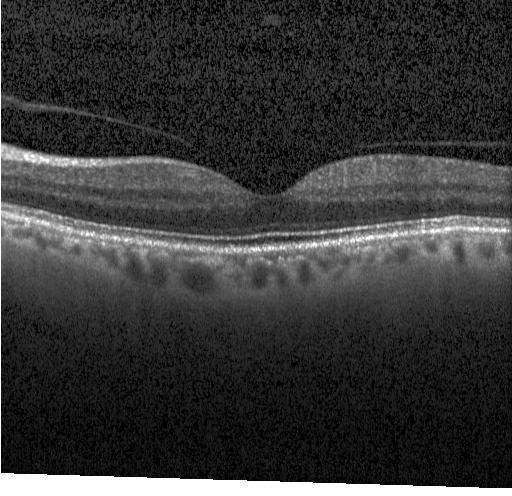

Retinal OCT cross-section. OCT finding: neither choroidal neovascularization, diabetic macular edema, nor drusen.